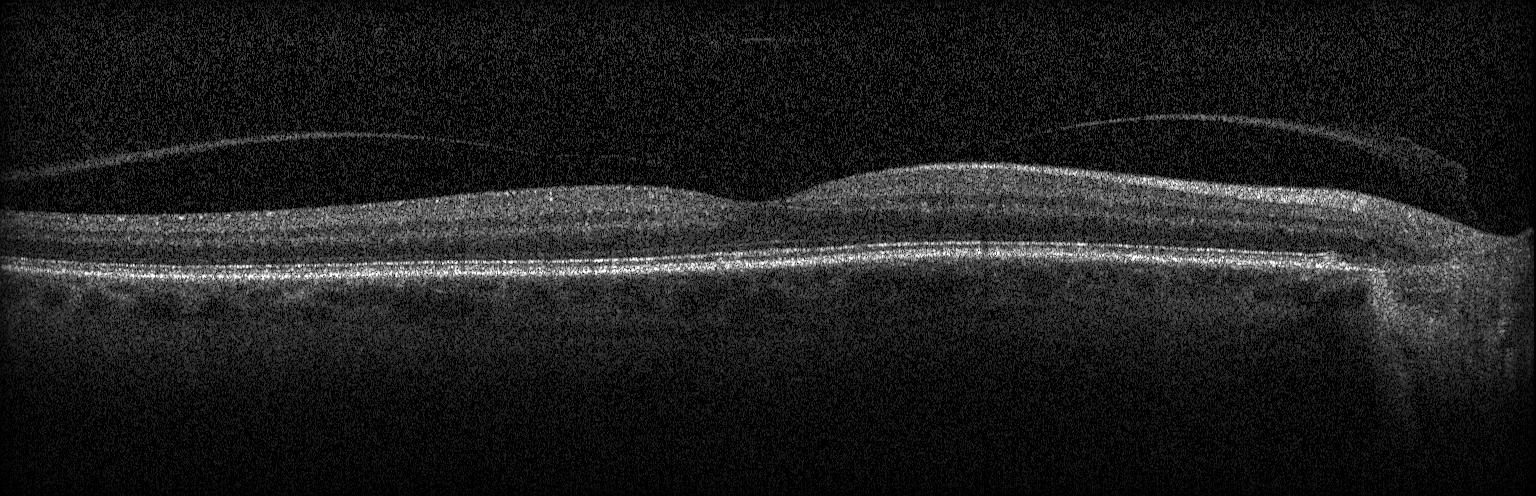
OCT B-scan showing no choroidal neovascularization, diabetic macular edema, or drusen.